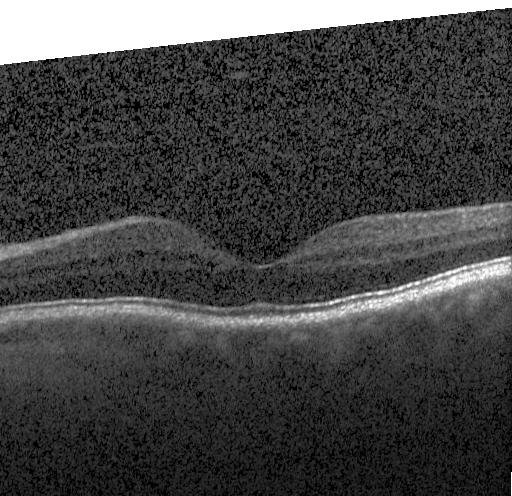 OCT finding: no choroidal neovascularization, no diabetic macular edema, and no drusen.